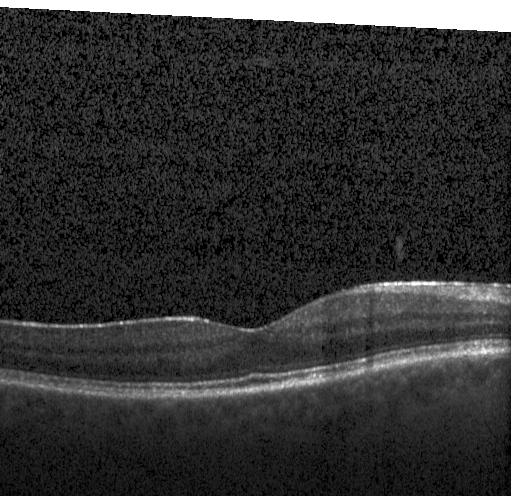
Centered on the fovea · SD-OCT · OCT line scan.
Diagnosis: neither choroidal neovascularization, diabetic macular edema, nor drusen.